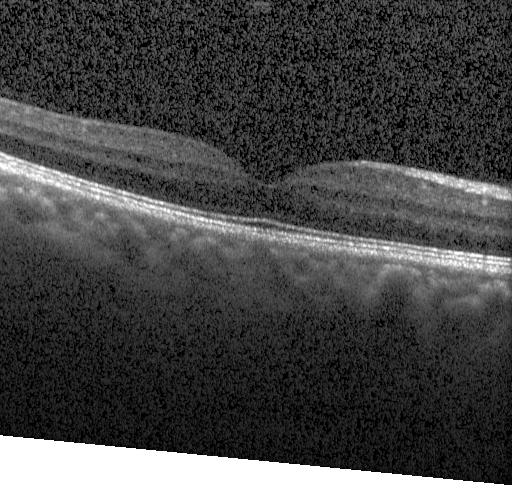
Fovea-centered; instrument: Heidelberg Spectralis; OCT line scan; spectral-domain optical coherence tomography.
Diagnosis: no CNV, no DME, and no drusen.